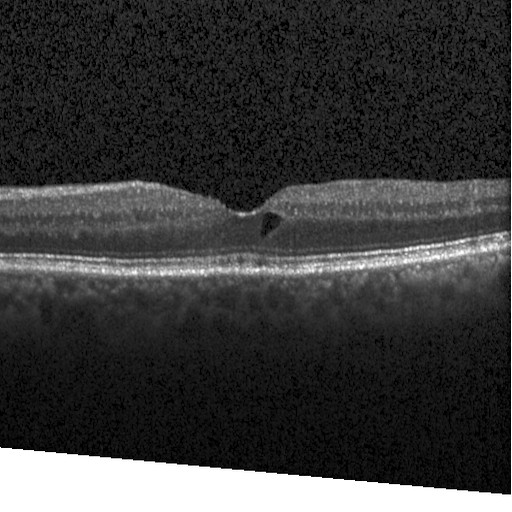 Heidelberg Spectralis · OCT B-scan.
Finding: diabetic macular edema (DME).